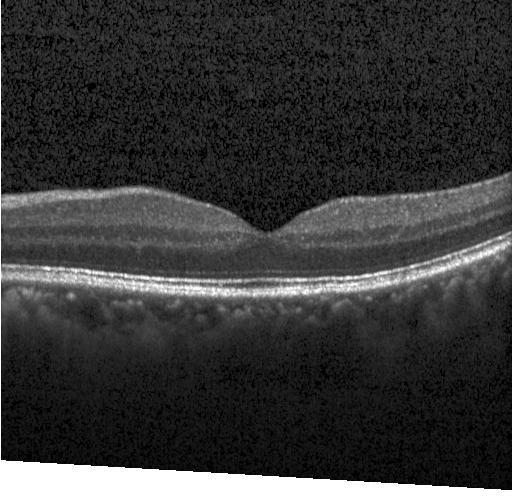
OCT scan showing no CNV, no DME, and no drusen.